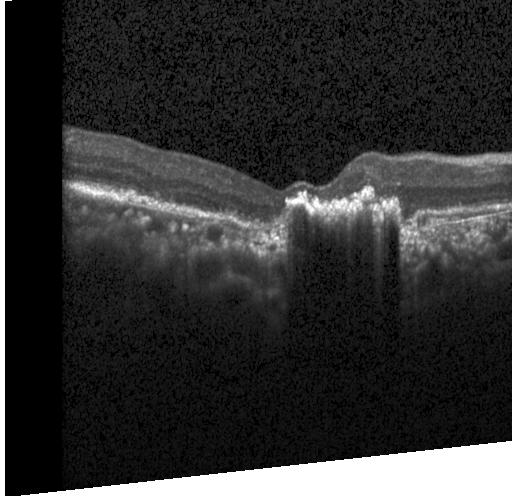 Diagnosis: CNV.